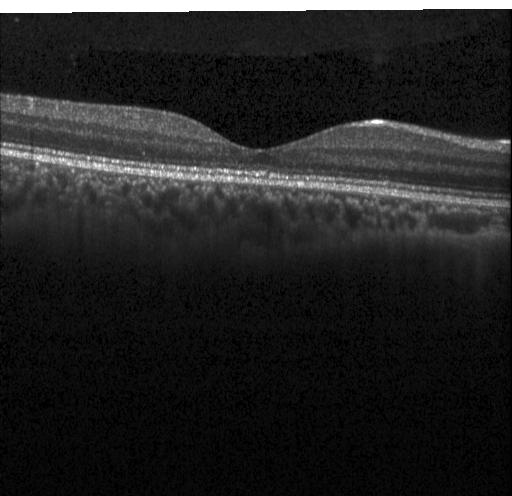 Spectral-domain optical coherence tomography. Retinal OCT cross-section. Horizontal scan through the fovea.
Finding: no choroidal neovascularization, no diabetic macular edema, and no drusen.